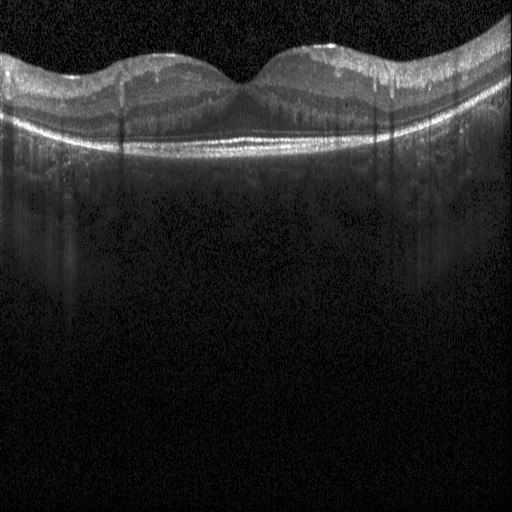

Finding: DME.